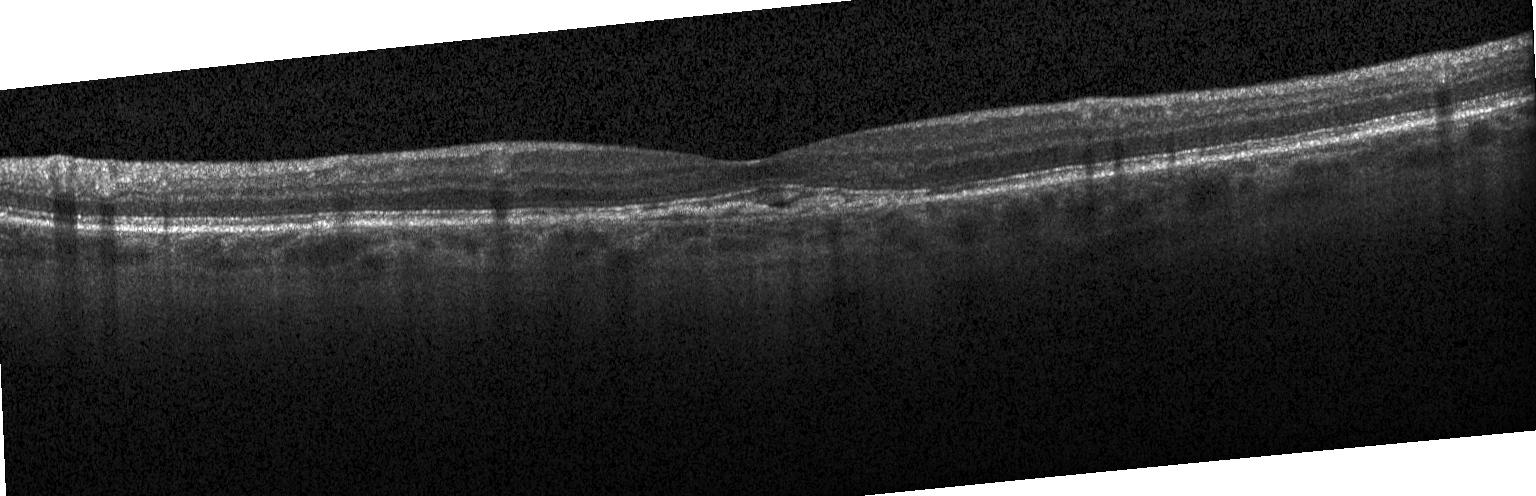
Retinal OCT cross-section; instrument: Heidelberg Spectralis; centered on the fovea — Impression: choroidal neovascularization (CNV).